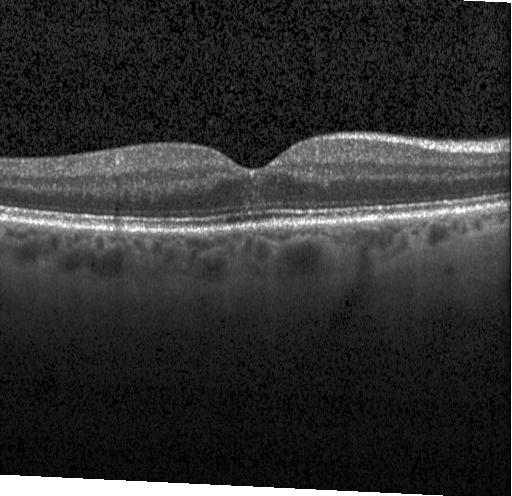 Retinal OCT cross-section; through the macula — The scan shows no CNV, no DME, and no drusen.